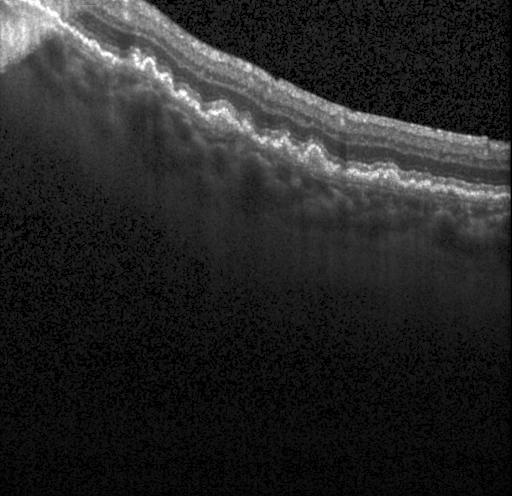
Spectral-domain optical coherence tomography, macular scan, acquired on a Heidelberg Spectralis, optical coherence tomography scan. A choroidal neovascular membrane.